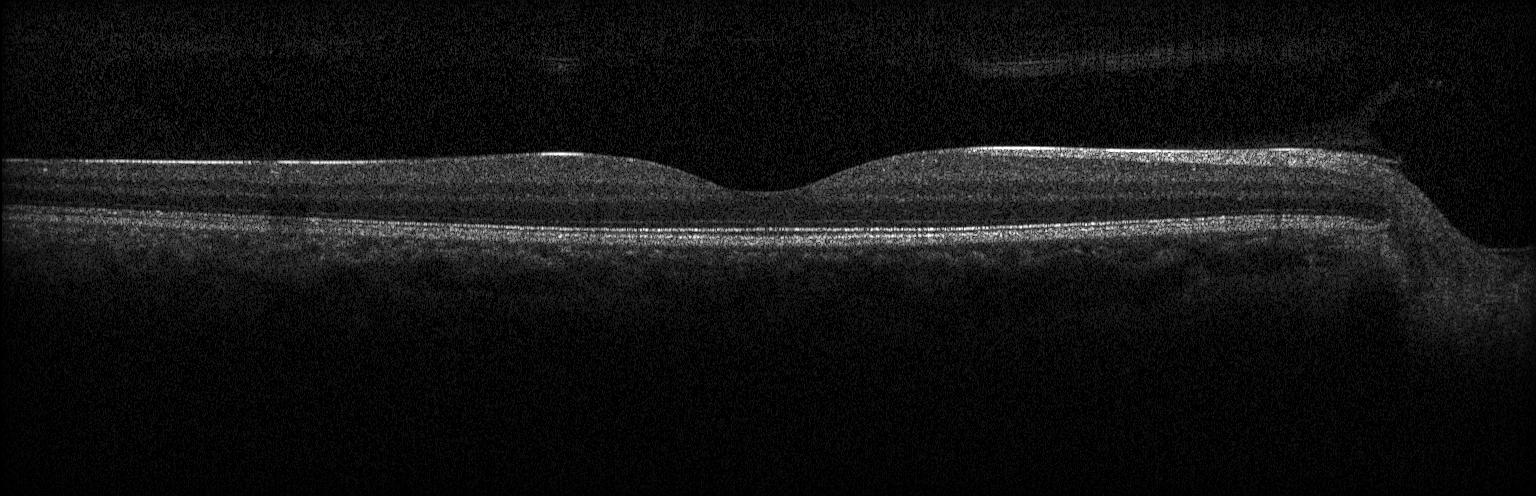

Finding: no choroidal neovascularization, no diabetic macular edema, and no drusen.